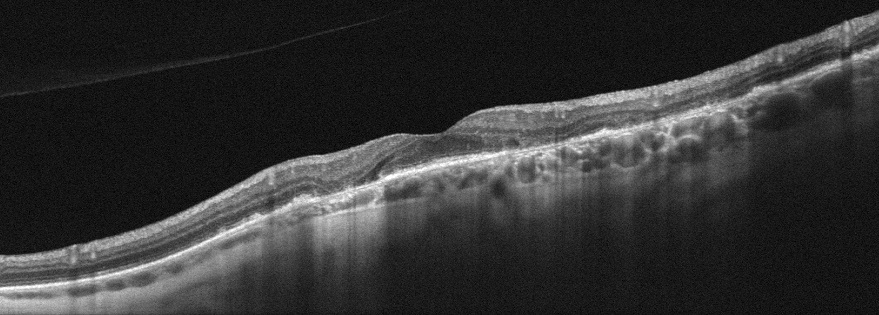 Dx: age-related macular degeneration.